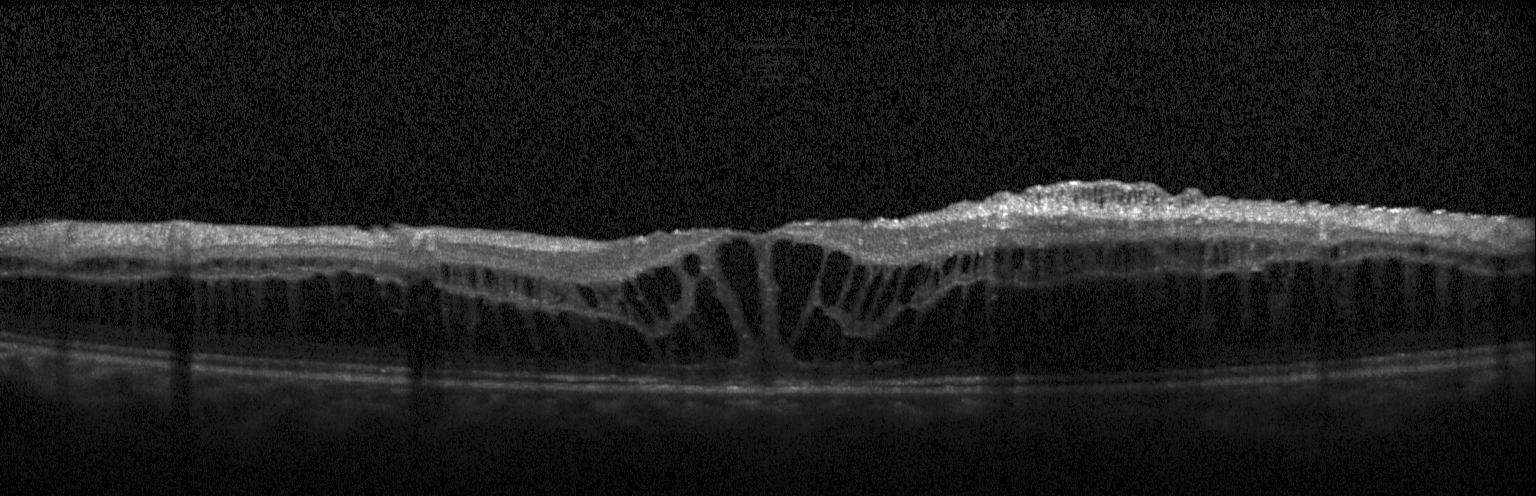

OCT line scan, Heidelberg Spectralis OCT system. Diagnosis: diabetic macular edema.